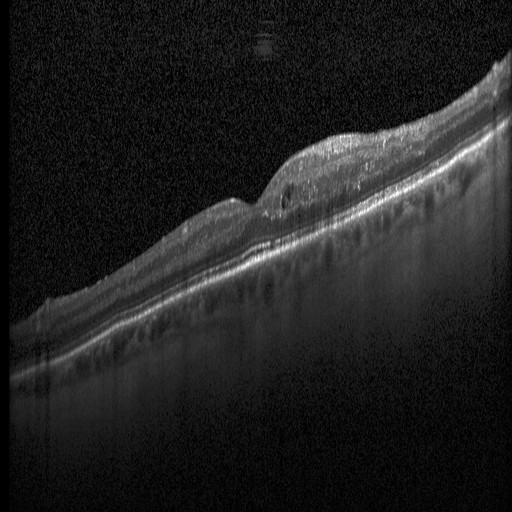
Dx: DME.